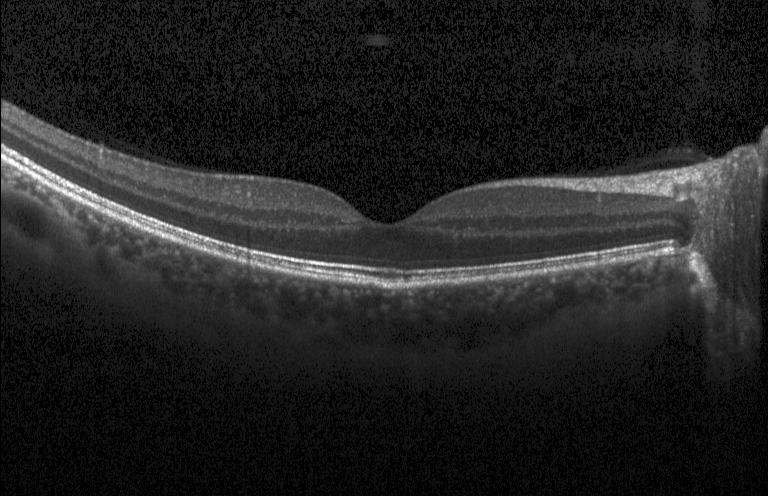
Optical coherence tomography B-scan; centered on the fovea
Impression: no choroidal neovascularization, diabetic macular edema, or drusen.